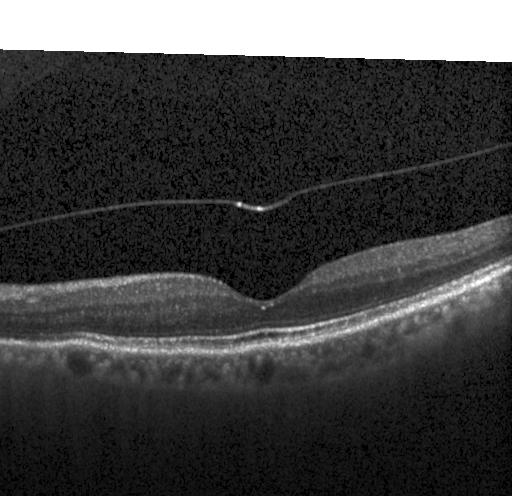 Optical coherence tomography scan. Horizontal scan through the fovea. Acquired on a Heidelberg Spectralis.
The scan shows no evidence of choroidal neovascularization, diabetic macular edema, or drusen.